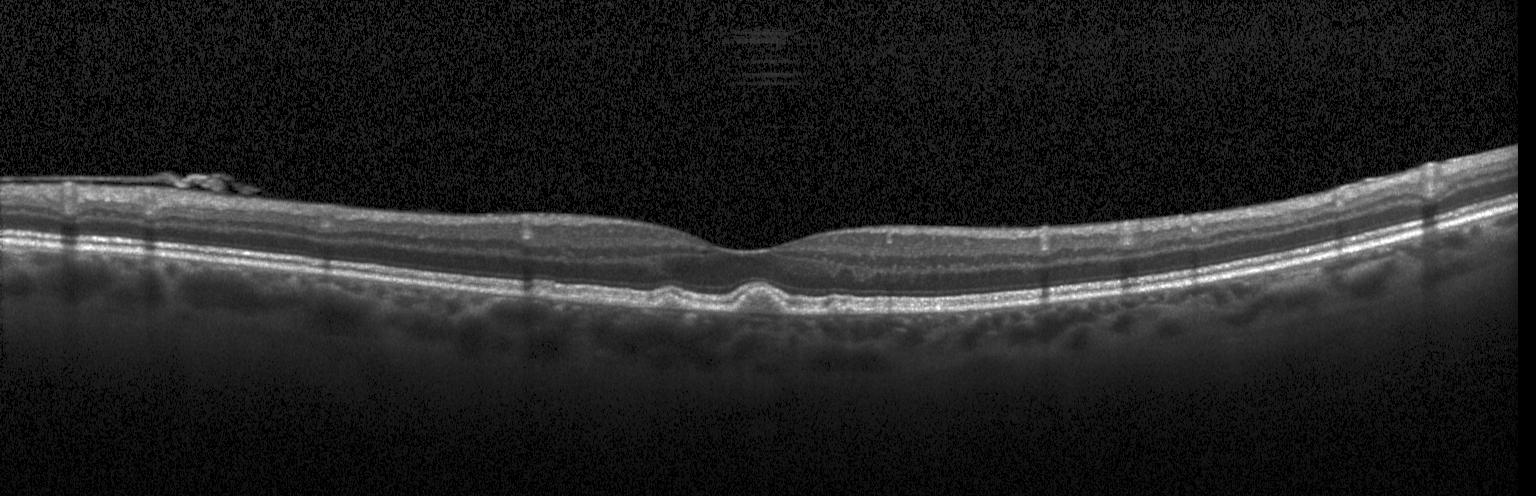
Retinal OCT B-scan · instrument: Heidelberg Spectralis · spectral-domain optical coherence tomography
Macular OCT: multiple drusen.